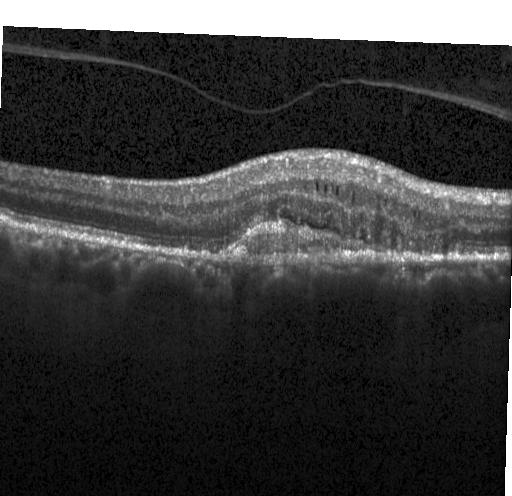 Finding: a choroidal neovascular membrane.